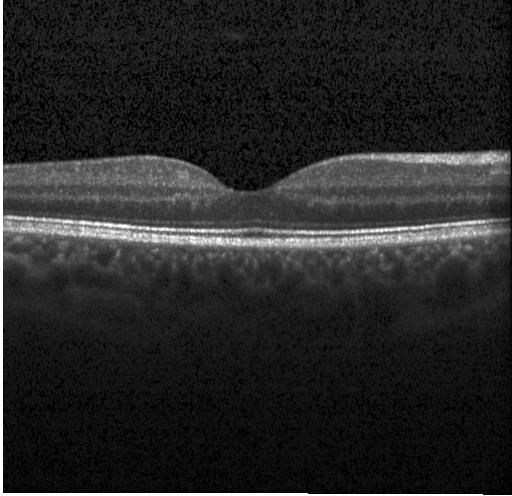
Impression: neither choroidal neovascularization, diabetic macular edema, nor drusen.